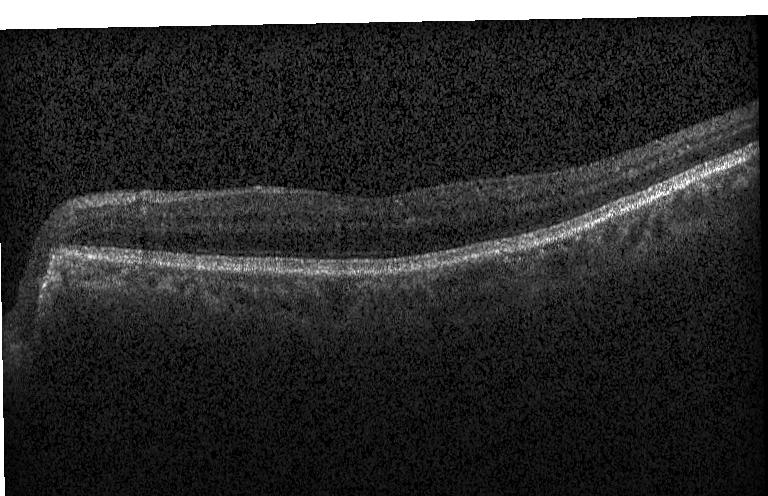

Macular OCT: neither CNV, DME, nor drusen.